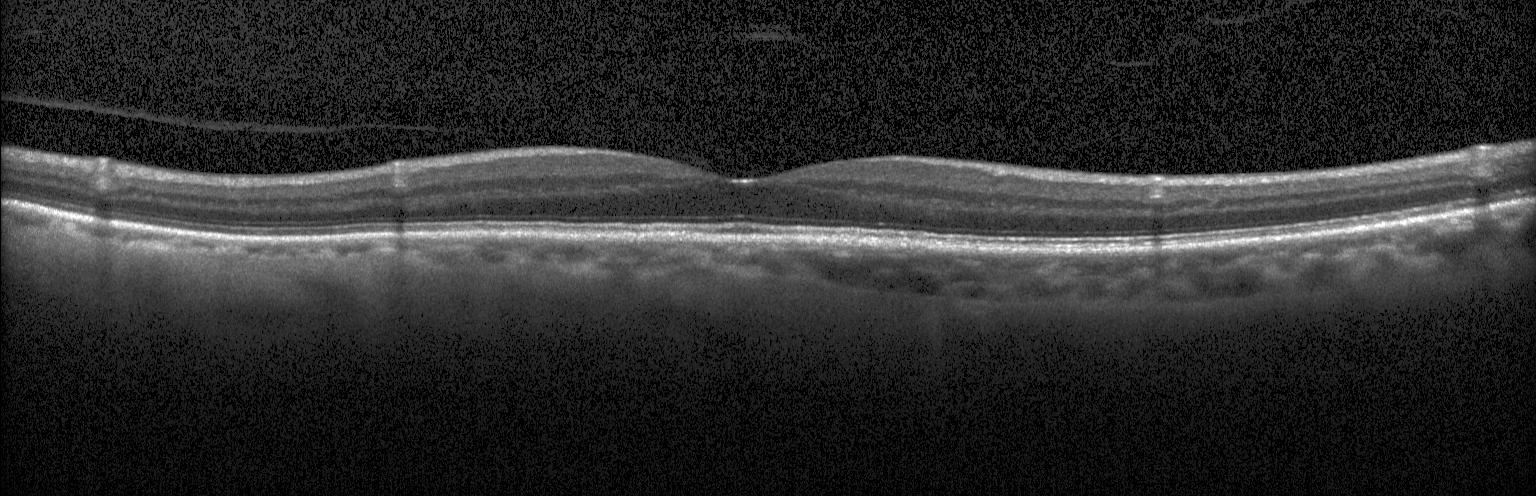 Optical coherence tomography B-scan
This B-scan demonstrates no CNV, no DME, and no drusen.